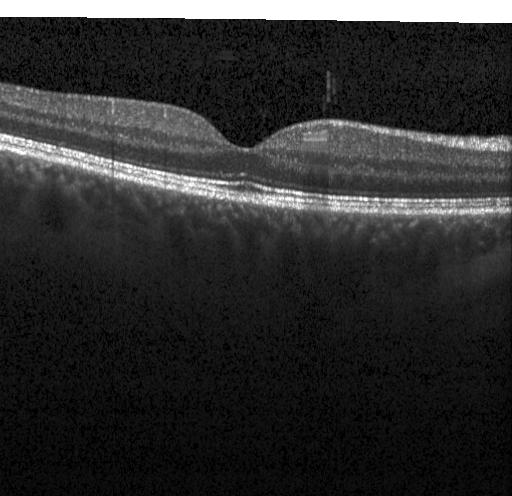

Optical coherence tomography scan.
No choroidal neovascularization, no diabetic macular edema, and no drusen.